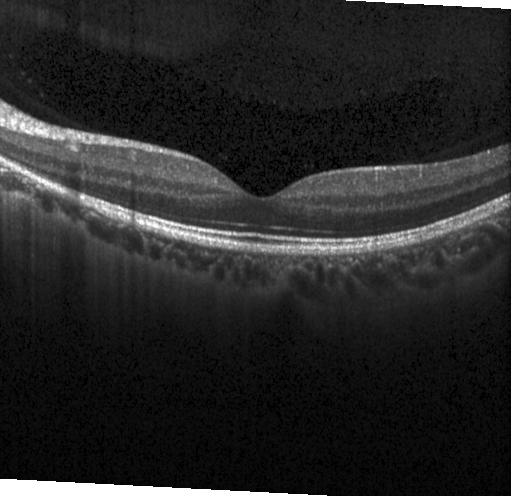

Retinal OCT cross-section
Diagnosis: neither CNV, DME, nor drusen.